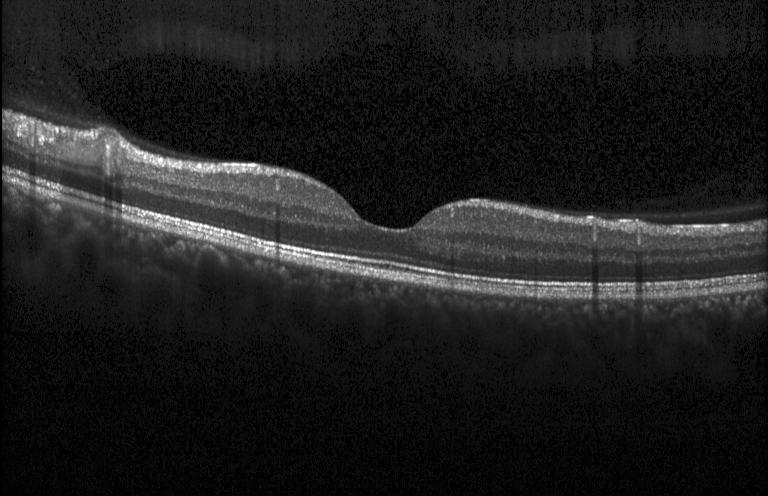
Retinal OCT cross-section showing no choroidal neovascularization, no diabetic macular edema, and no drusen.